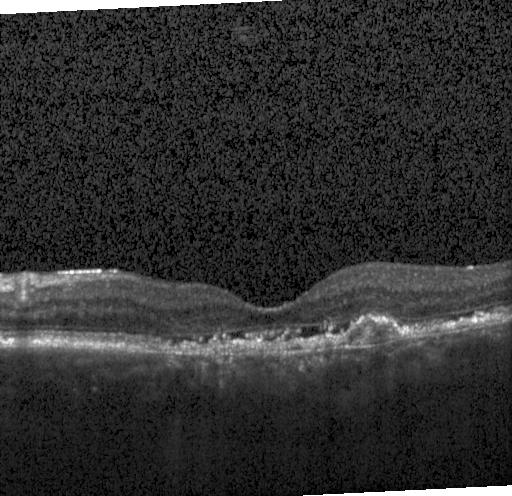

Finding: CNV.